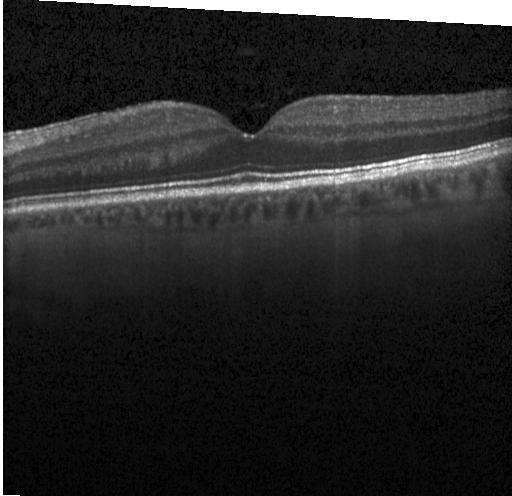

Assessment: no CNV, DME, or drusen.